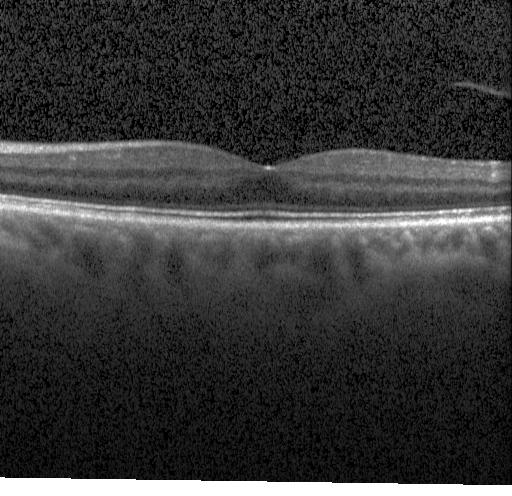
Macular OCT: no evidence of choroidal neovascularization, diabetic macular edema, or drusen.